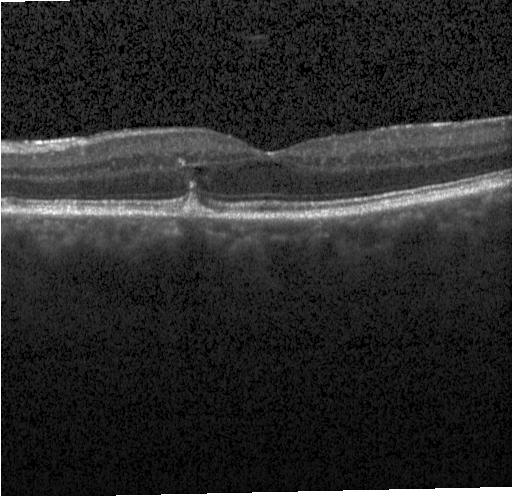

OCT line scan · Heidelberg Spectralis OCT system — Finding: a choroidal neovascular membrane.